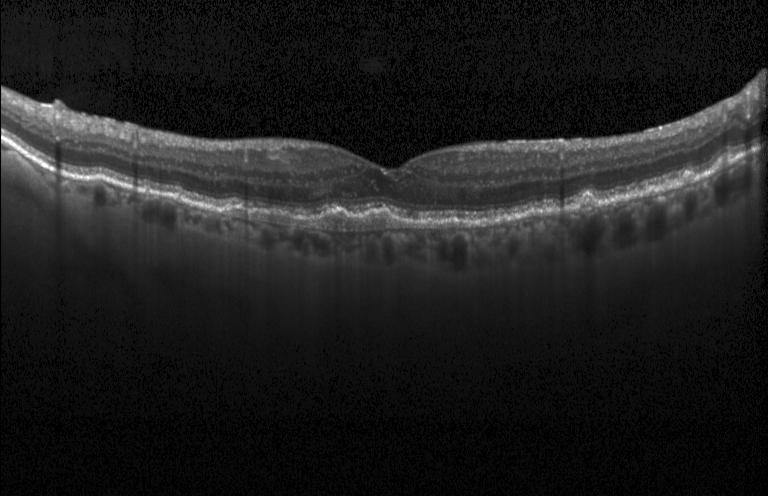 Spectral-domain optical coherence tomography. Optical coherence tomography scan. Heidelberg Spectralis OCT system. Finding: a choroidal neovascular membrane.